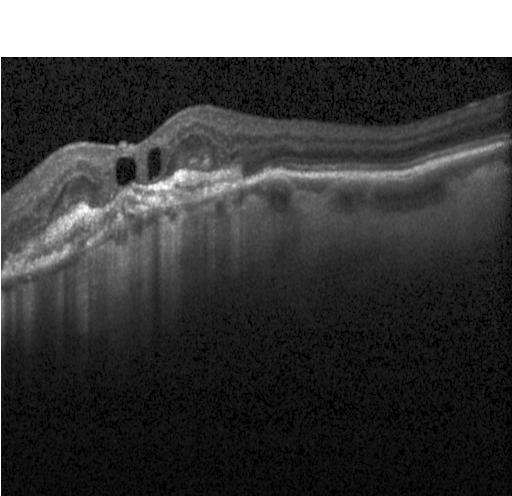
Heidelberg Spectralis OCT system; retinal OCT cross-section. The scan shows a choroidal neovascular membrane.